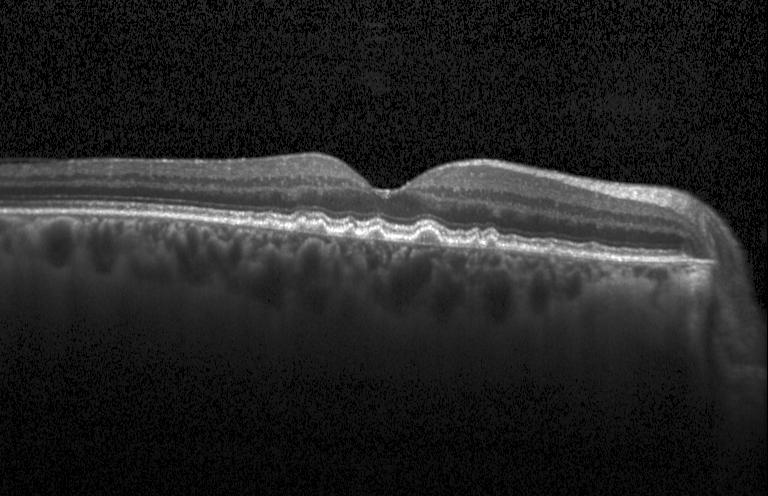

Retinal OCT B-scan; Heidelberg Spectralis
Dx: multiple drusen.